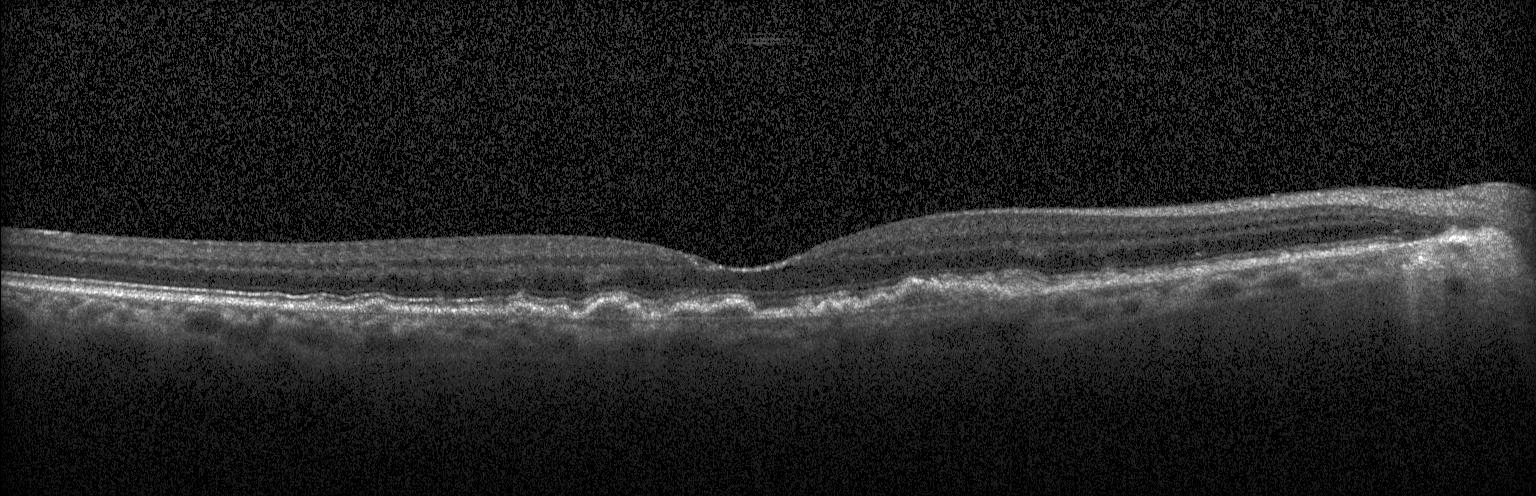

Through the macula, OCT B-scan, instrument: Heidelberg Spectralis, SD-OCT.
Assessment: multiple drusen.